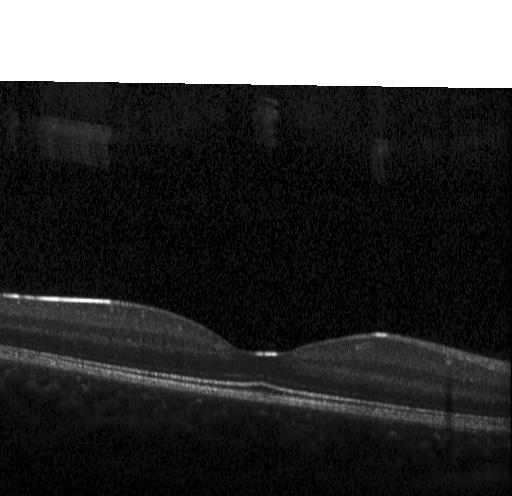 Retinal OCT cross-section — Impression: neither choroidal neovascularization, diabetic macular edema, nor drusen.